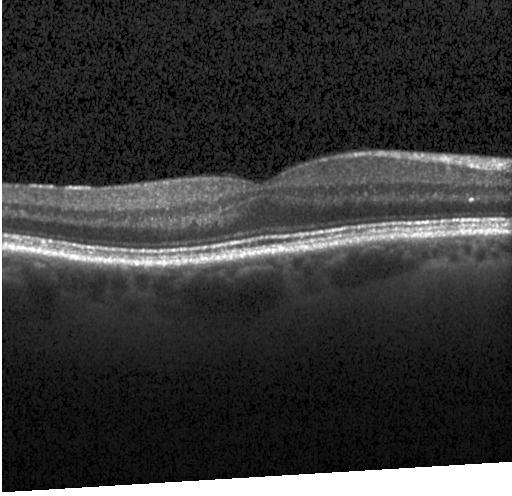
OCT finding: no evidence of CNV, DME, or drusen.